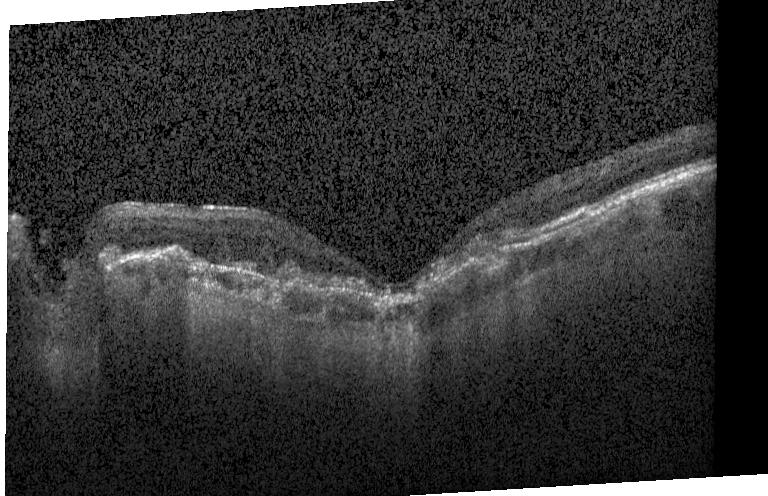

OCT B-scan. Heidelberg Spectralis OCT system. Spectral-domain OCT.
CNV.